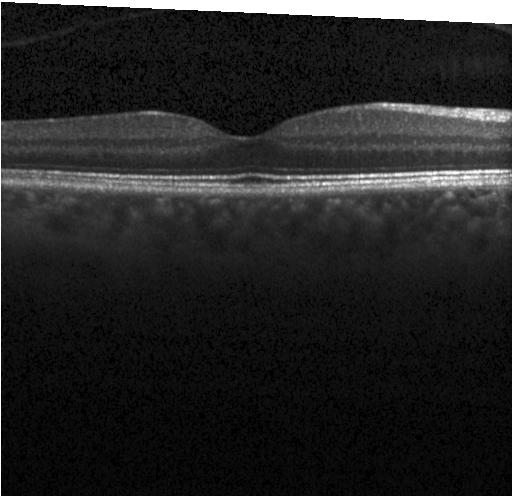
OCT B-scan
This B-scan demonstrates no evidence of choroidal neovascularization, diabetic macular edema, or drusen.